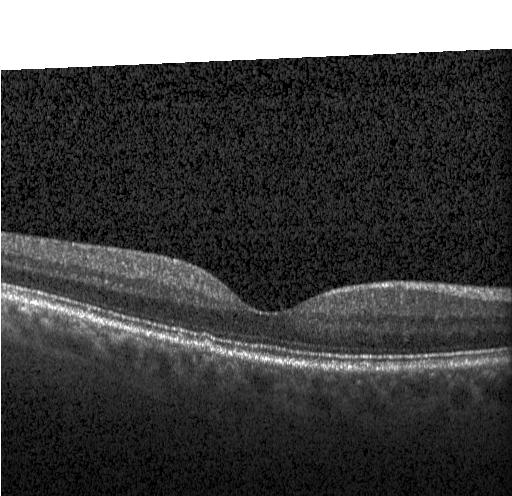

Optical coherence tomography scan; spectral-domain optical coherence tomography. Diagnosis: no CNV, DME, or drusen.